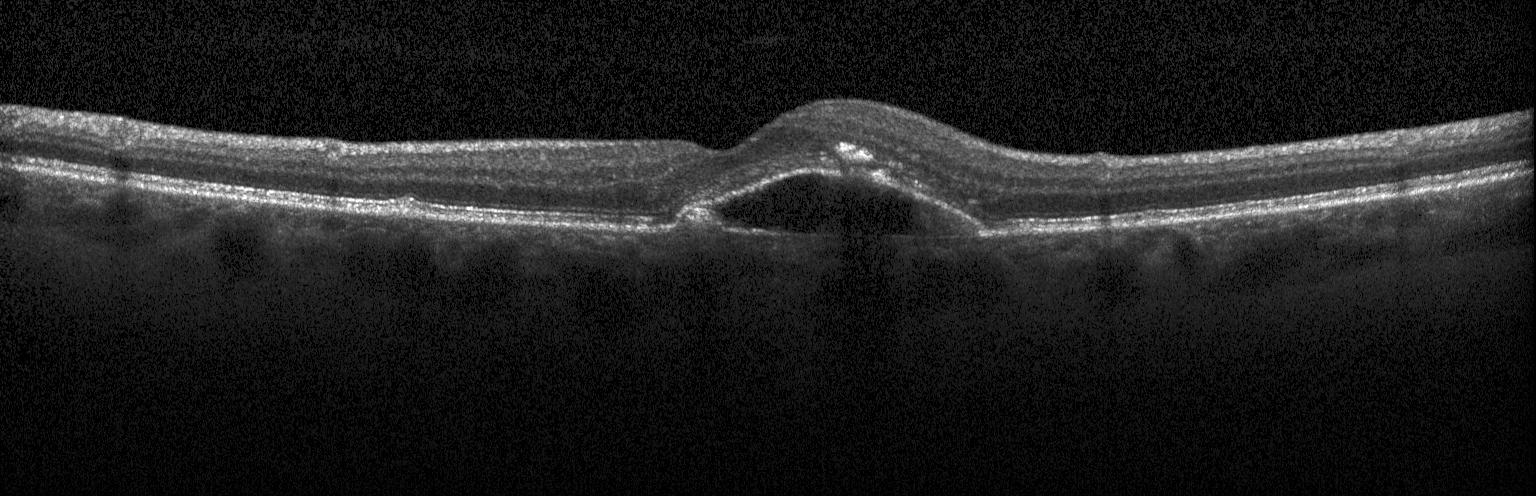

Retinal OCT B-scan. Horizontal scan through the fovea — OCT finding: CNV.